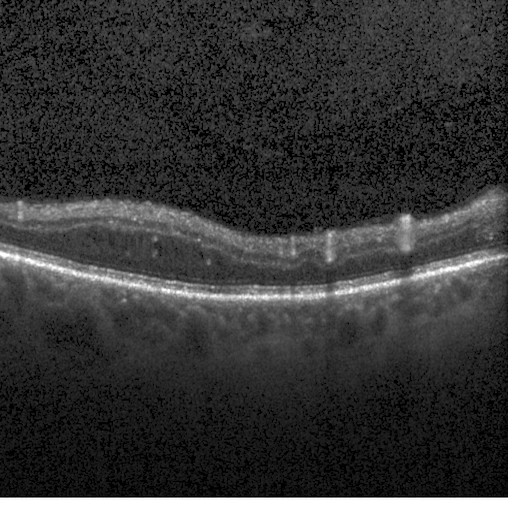

Optical coherence tomography B-scan. Heidelberg Spectralis. Horizontal scan through the fovea. Spectral-domain optical coherence tomography.
OCT finding: diabetic macular edema (DME).